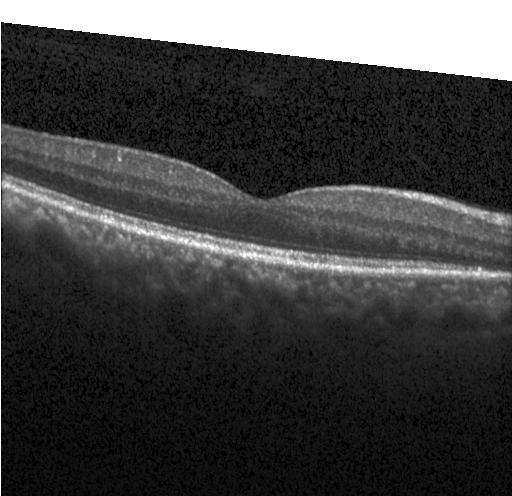 Impression: no choroidal neovascularization, diabetic macular edema, or drusen.